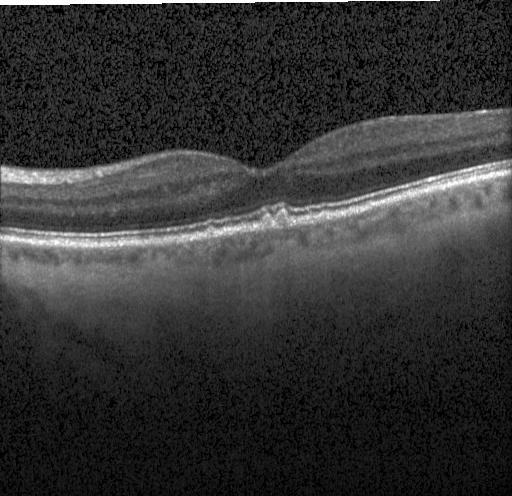

This B-scan demonstrates multiple drusen.